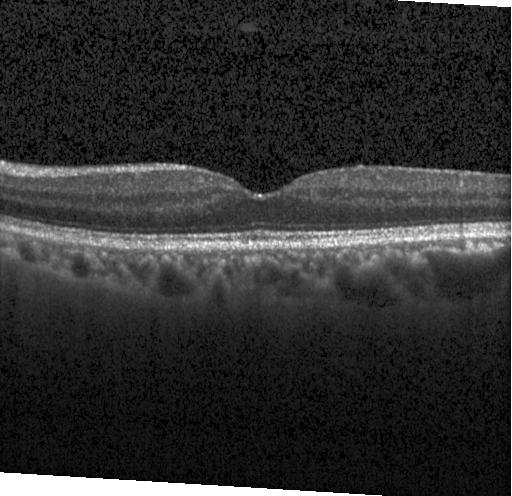 Diagnosis: neither choroidal neovascularization, diabetic macular edema, nor drusen.